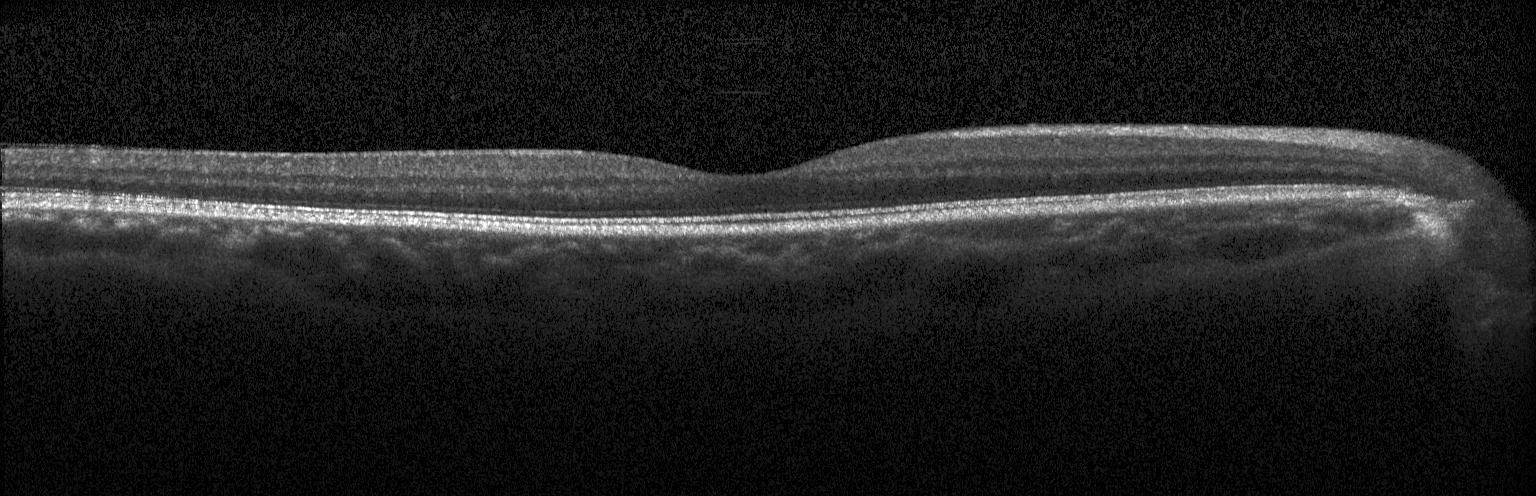
OCT scan showing no choroidal neovascularization, no diabetic macular edema, and no drusen.